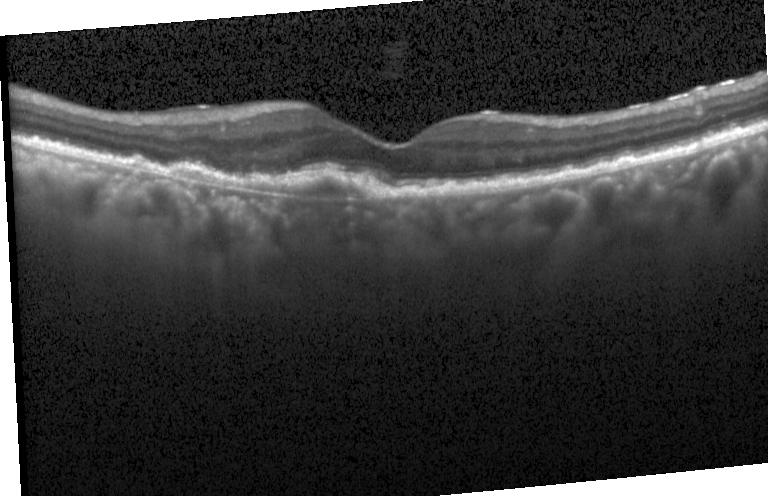 Finding: choroidal neovascularization.